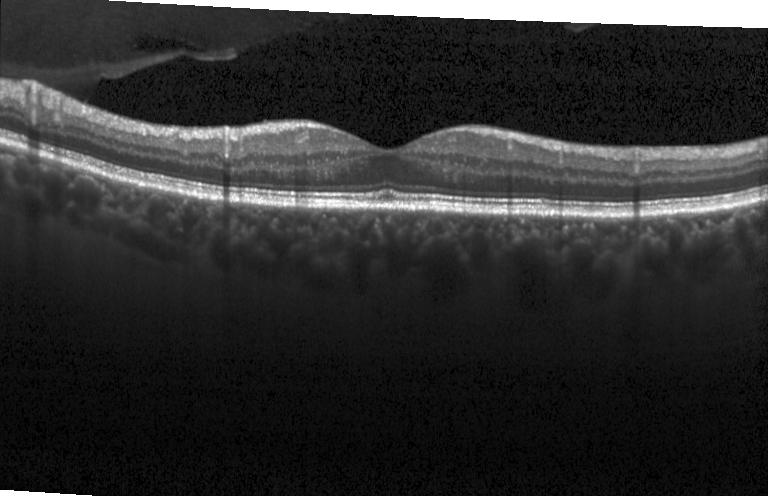
Instrument: Heidelberg Spectralis. Macular scan. Spectral-domain optical coherence tomography. OCT line scan
Assessment: neither CNV, DME, nor drusen.